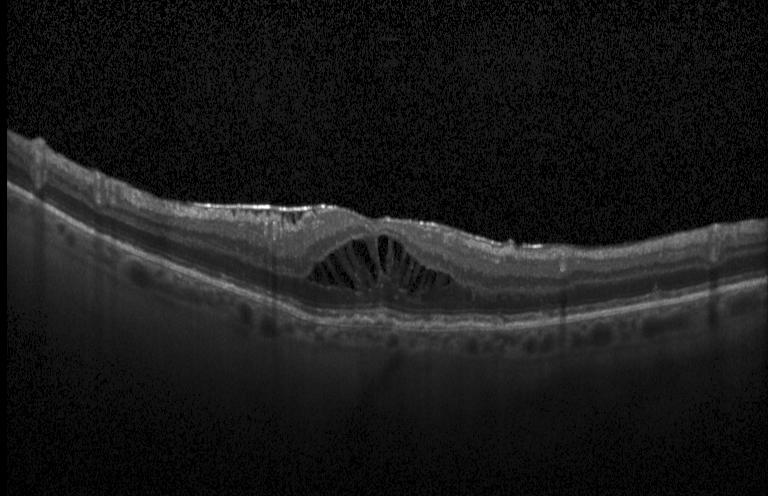 Retinal OCT cross-section · Heidelberg Spectralis
This B-scan demonstrates diabetic macular edema.